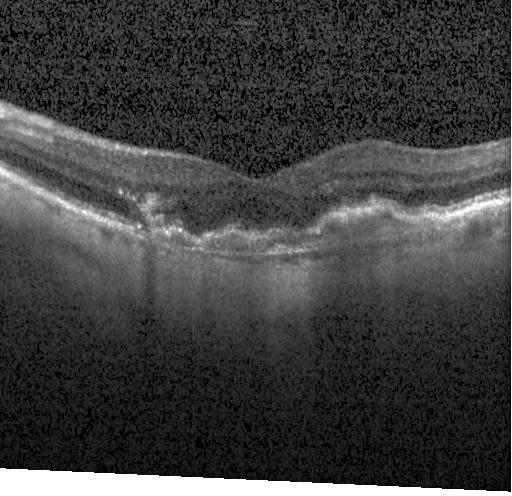 OCT B-scan showing a choroidal neovascular membrane.